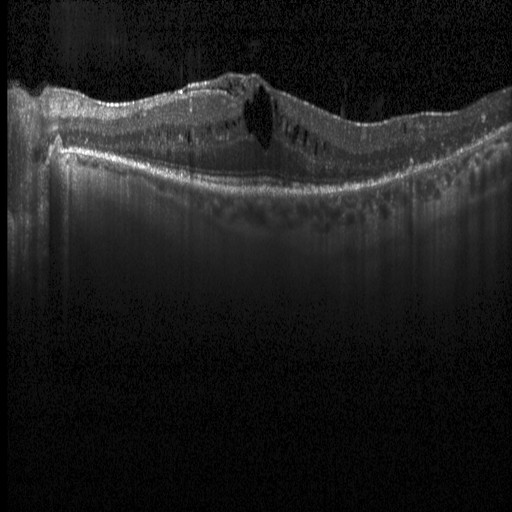 Macular OCT: diabetic macular edema (DME).